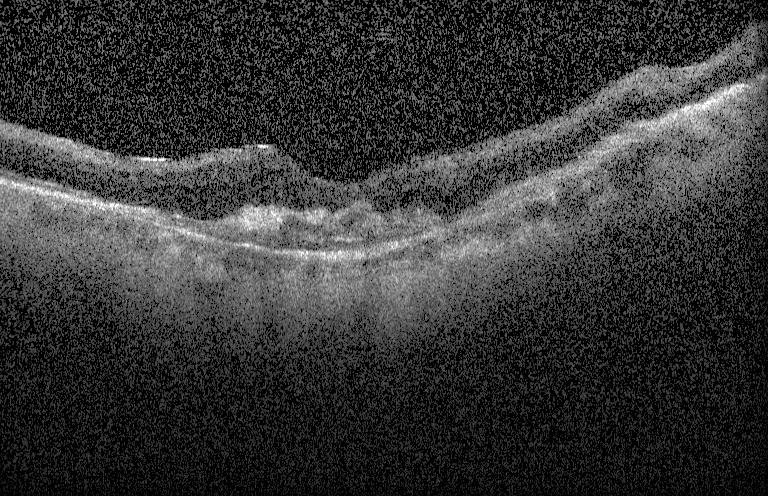 Acquired on a Heidelberg Spectralis · spectral-domain OCT · optical coherence tomography B-scan · macular scan.
Macular OCT: CNV.